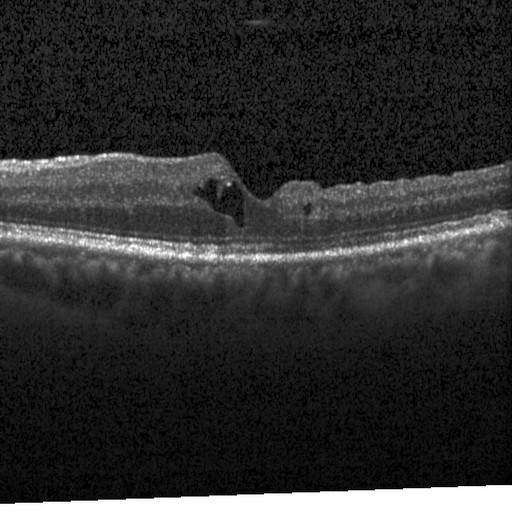 Horizontal scan through the fovea. Spectral-domain OCT. Acquired on a Heidelberg Spectralis. OCT B-scan — The scan shows DME.